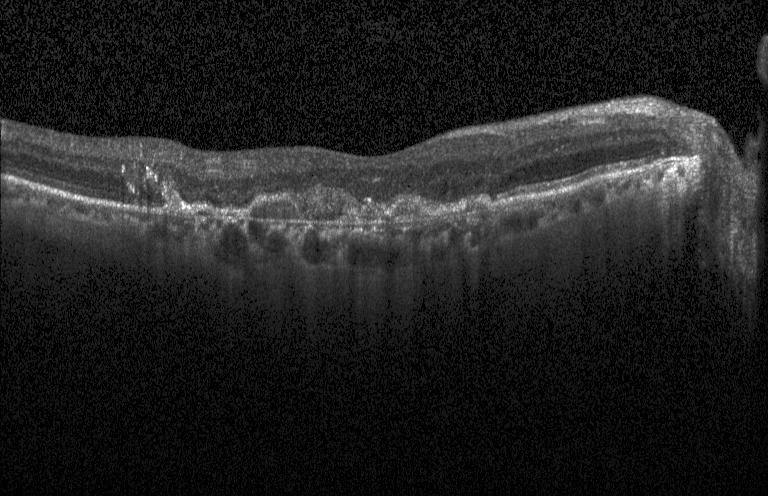

Spectral-domain optical coherence tomography. Retinal OCT cross-section.
Macular OCT: a choroidal neovascular membrane.